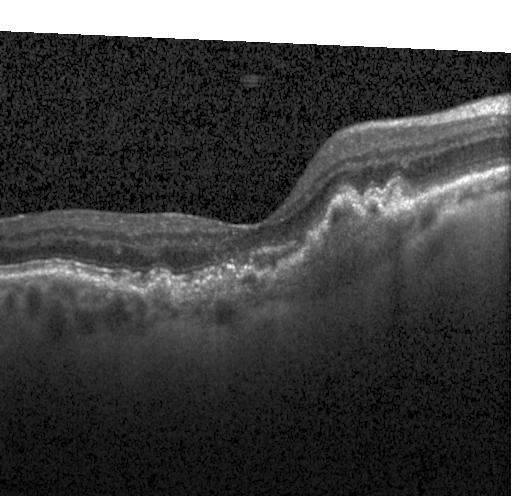 Centered on the fovea. Heidelberg Spectralis. OCT line scan
Impression: CNV.